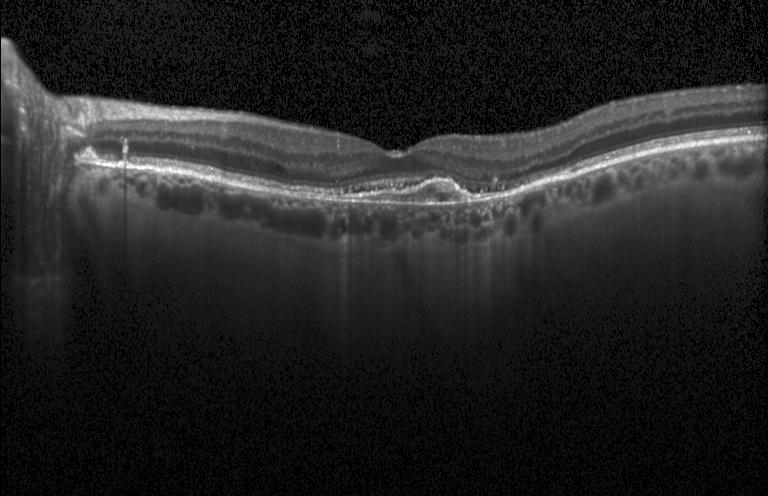 Spectral-domain optical coherence tomography; macular scan; optical coherence tomography scan.
This B-scan demonstrates choroidal neovascularization.